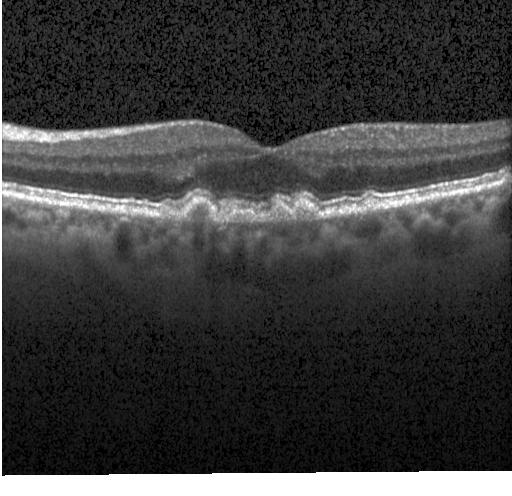
Fovea-centered. Spectral-domain OCT. Retinal OCT cross-section
The scan shows multiple drusen.